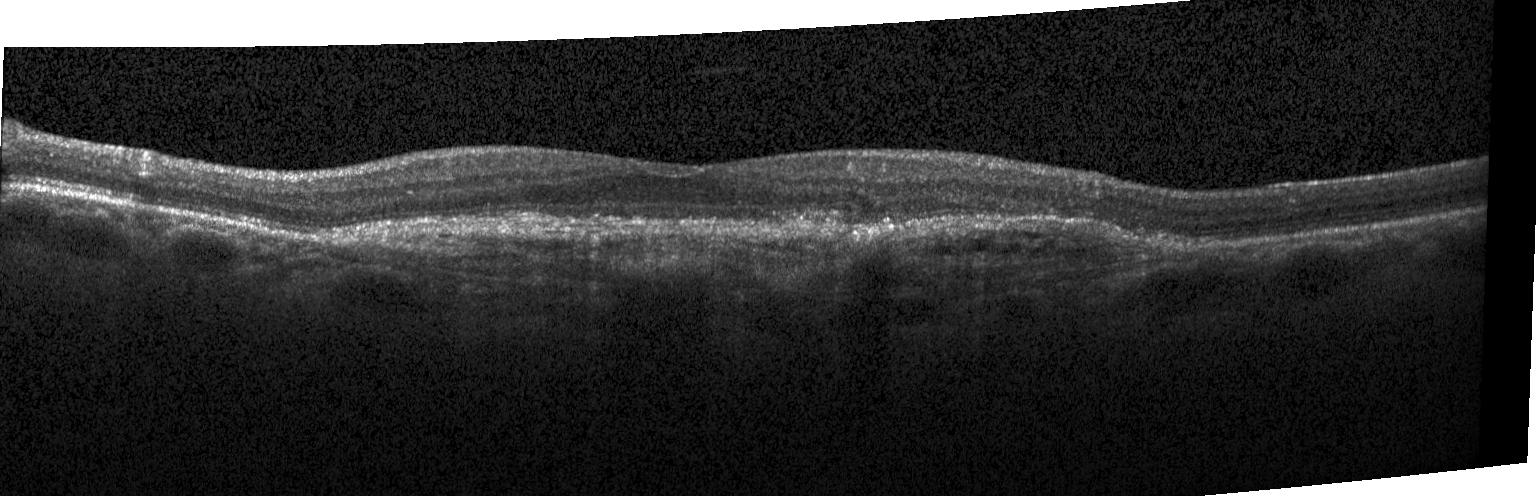 Retinal OCT B-scan.
Finding: a choroidal neovascular membrane.